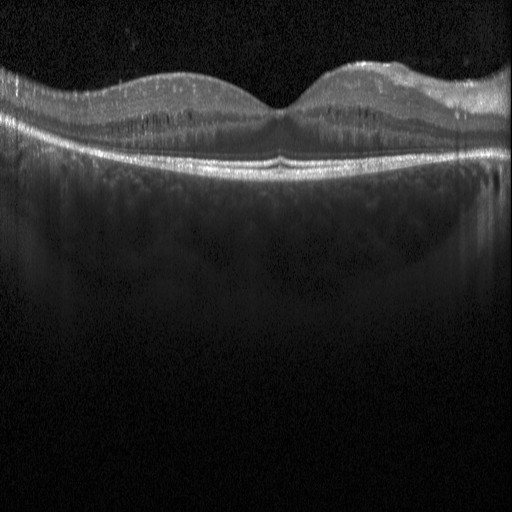 Finding: diabetic macular edema (DME).